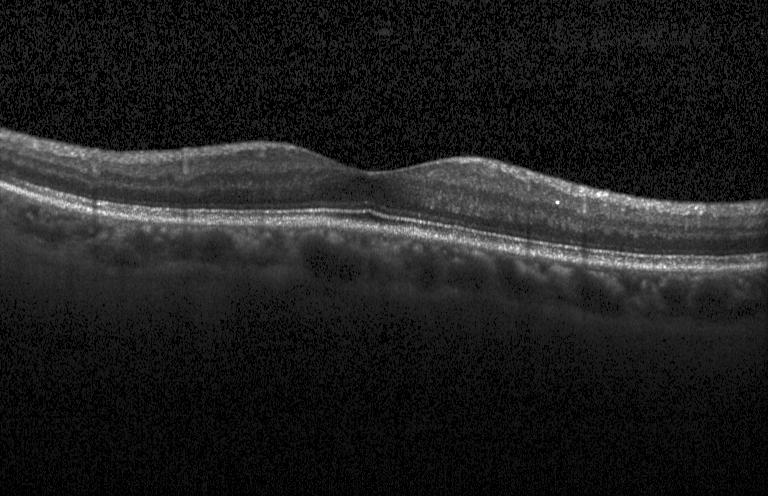 Finding: no choroidal neovascularization, no diabetic macular edema, and no drusen.